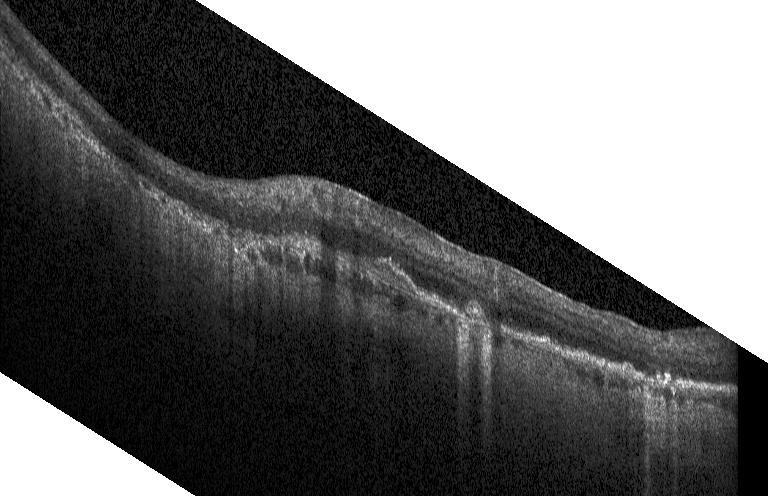

OCT B-scan. This B-scan demonstrates choroidal neovascularization (CNV).